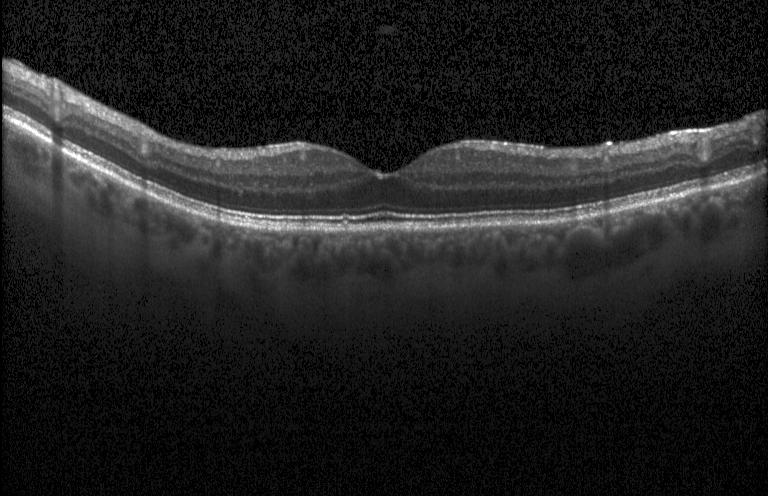
OCT B-scan. Diagnosis: neither CNV, DME, nor drusen.